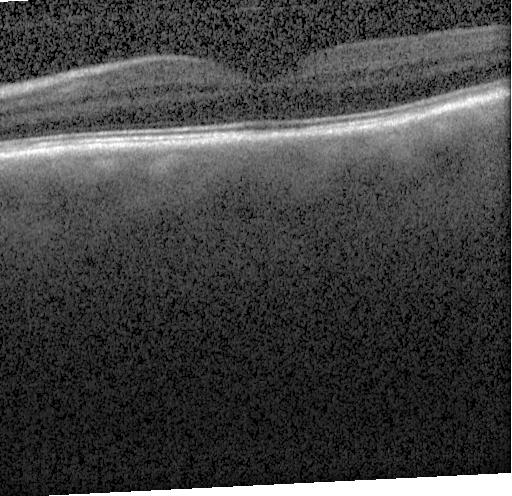 Diagnosis: no evidence of CNV, DME, or drusen.